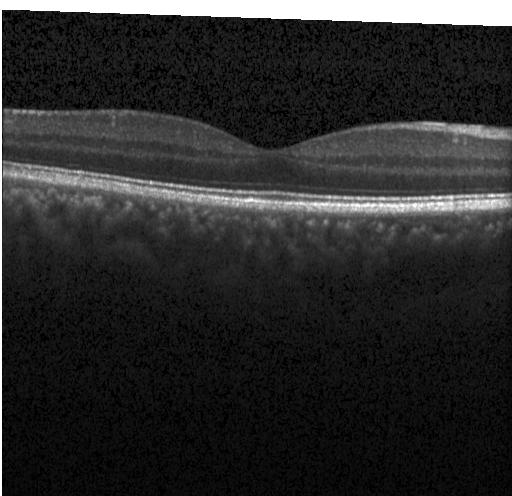 Impression: no evidence of choroidal neovascularization, diabetic macular edema, or drusen.